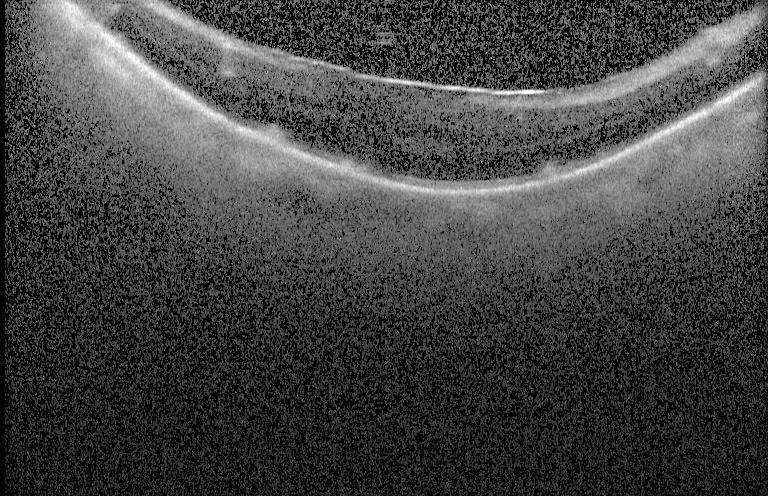

Instrument: Heidelberg Spectralis, optical coherence tomography B-scan.
Assessment: sub-RPE drusenoid deposits.